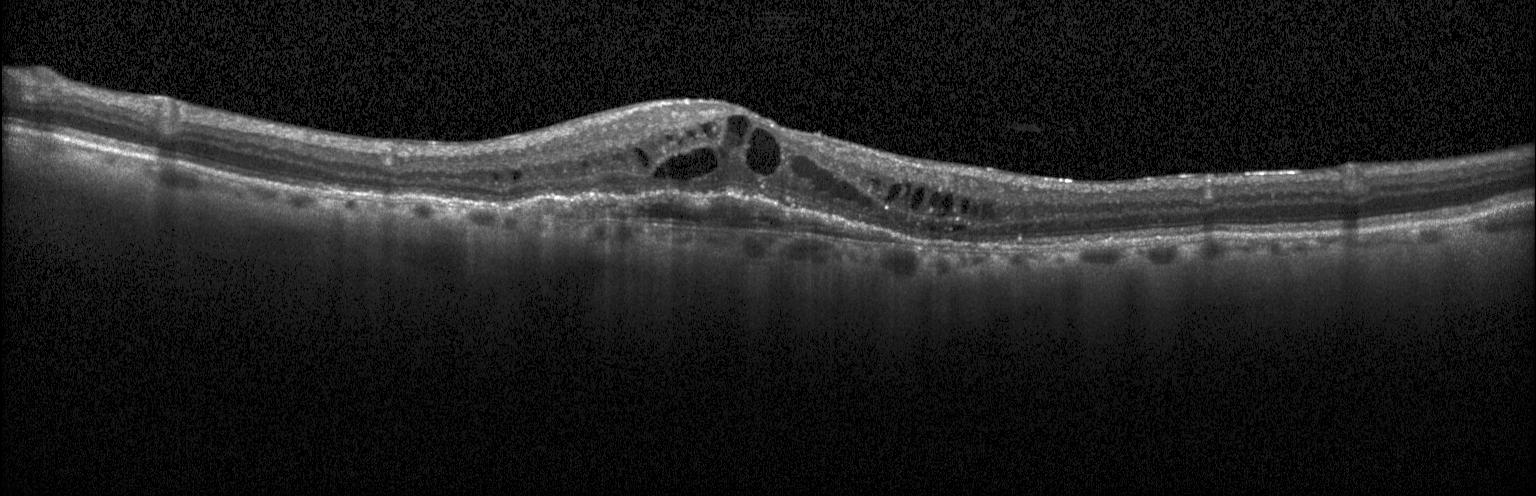

Optical coherence tomography B-scan; Heidelberg Spectralis OCT system; spectral-domain optical coherence tomography.
OCT finding: a choroidal neovascular membrane.